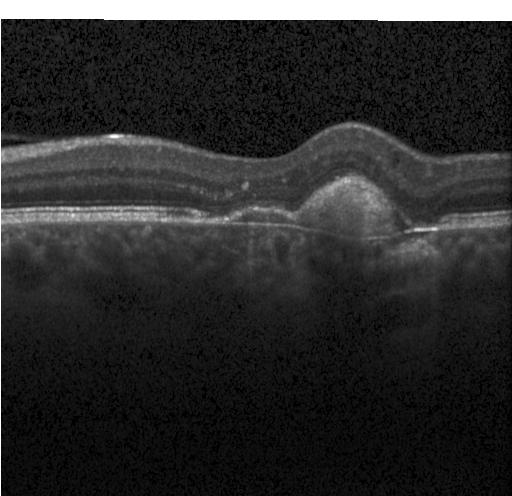 OCT line scan; SD-OCT
A choroidal neovascular membrane.